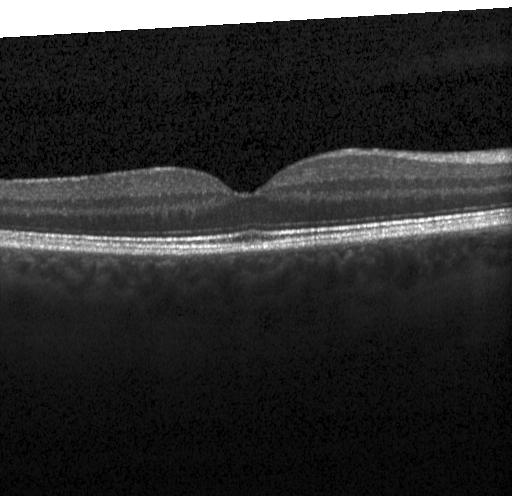
Retinal OCT cross-section.
Assessment: no CNV, DME, or drusen.